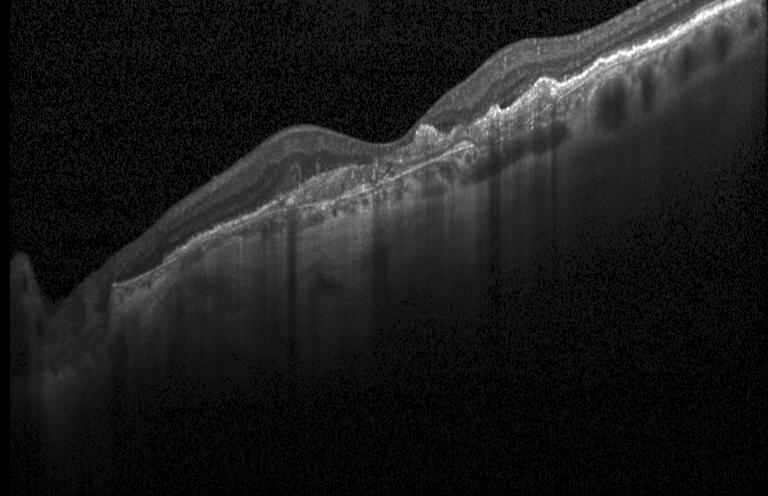
OCT B-scan, spectral-domain OCT, Heidelberg Spectralis OCT system.
Impression: choroidal neovascularization (CNV).